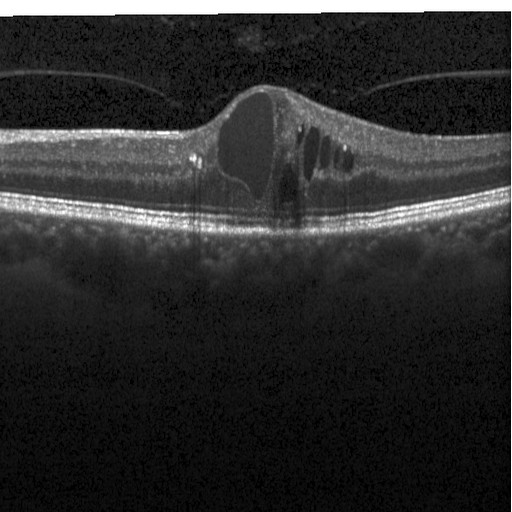 OCT B-scan · horizontal scan through the fovea — OCT finding: diabetic macular edema (DME).